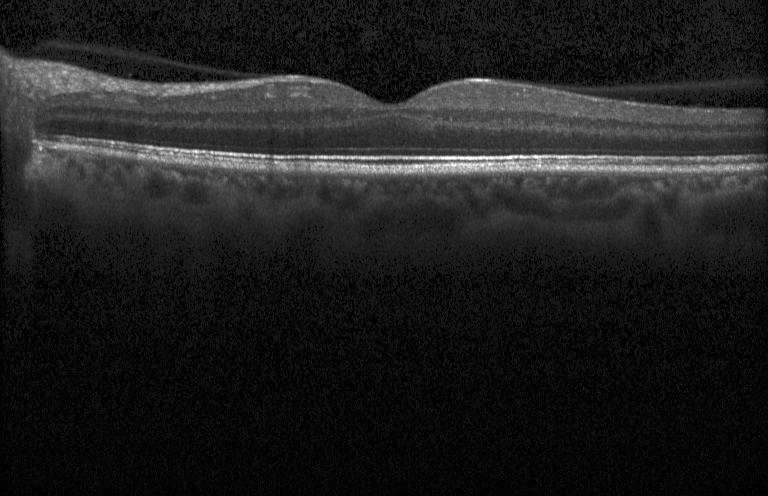 Spectral-domain OCT; instrument: Heidelberg Spectralis; horizontal scan through the fovea; retinal OCT B-scan
This B-scan demonstrates neither CNV, DME, nor drusen.